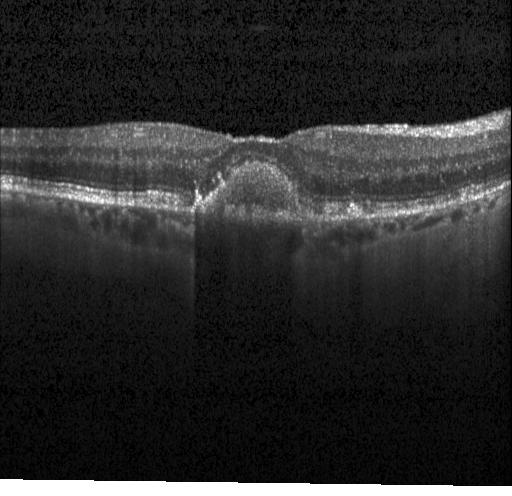
Diagnosis: a choroidal neovascular membrane.